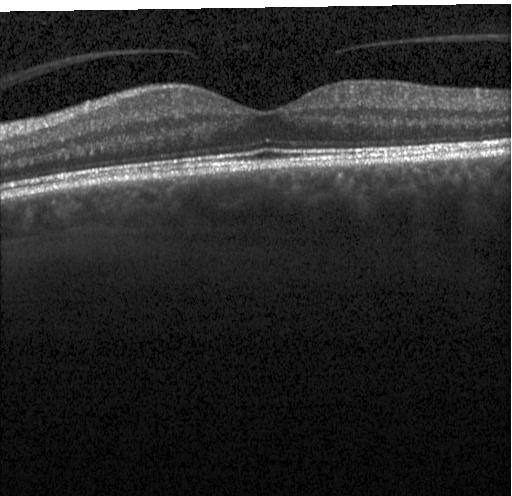
Impression: no CNV, no DME, and no drusen.